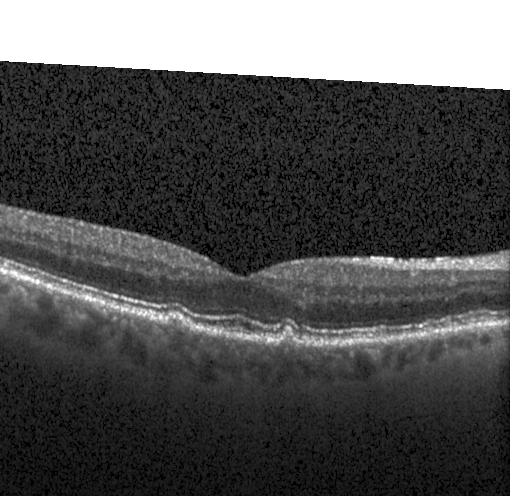 Optical coherence tomography scan. Heidelberg Spectralis. Spectral-domain optical coherence tomography — Impression: multiple drusen.